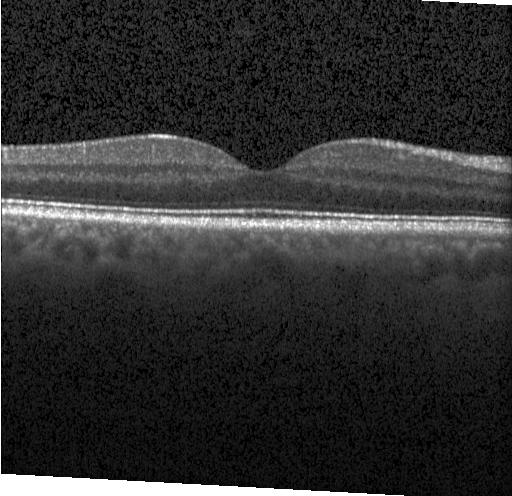
Fovea-centered, SD-OCT, Heidelberg Spectralis, optical coherence tomography scan. Finding: no choroidal neovascularization, no diabetic macular edema, and no drusen.